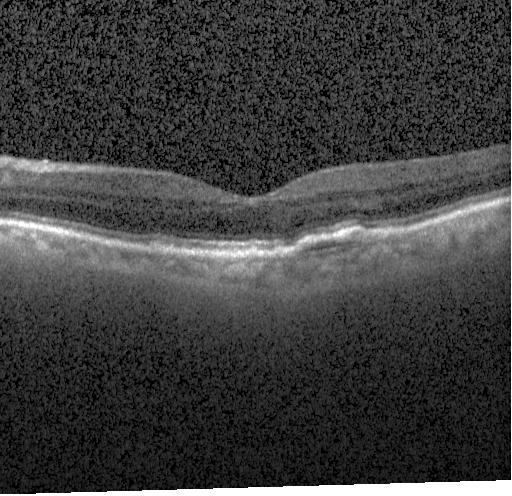 Diagnosis: a choroidal neovascular membrane.